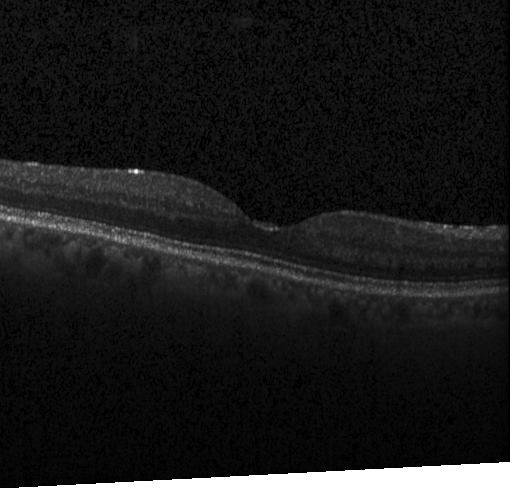

Optical coherence tomography scan. Diagnosis: no choroidal neovascularization, no diabetic macular edema, and no drusen.